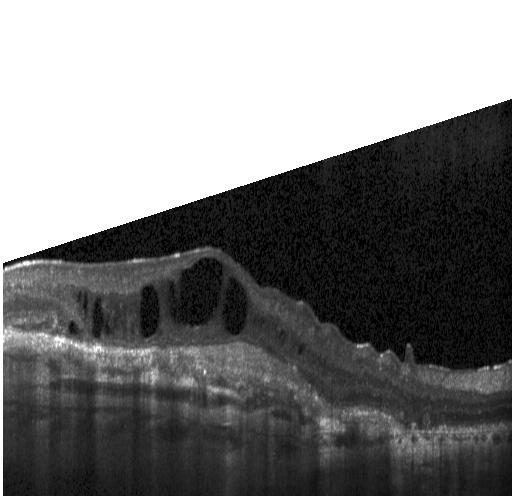
Retinal OCT cross-section showing a choroidal neovascular membrane.